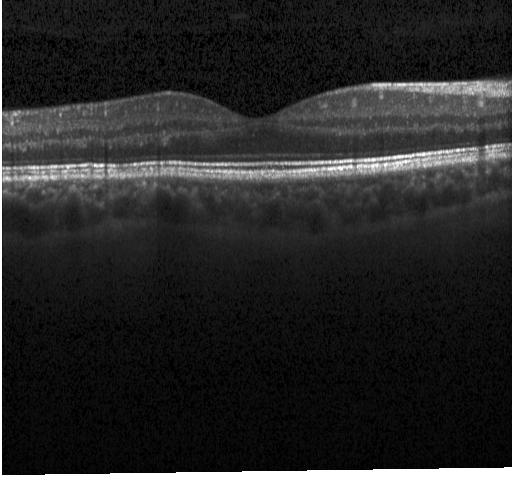 Optical coherence tomography B-scan.
Finding: no CNV, DME, or drusen.